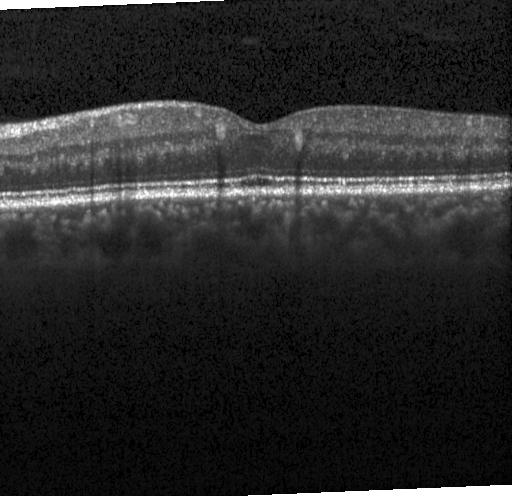 Optical coherence tomography scan · acquired on a Heidelberg Spectralis · through the macula · SD-OCT.
Diagnosis: no evidence of choroidal neovascularization, diabetic macular edema, or drusen.